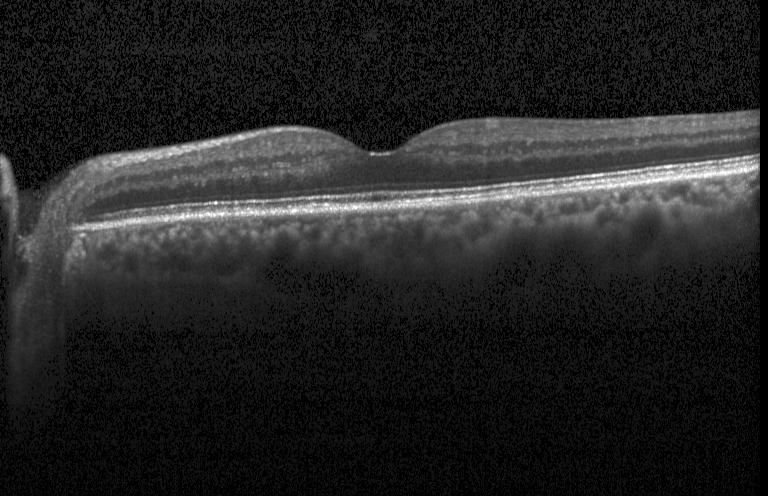 Retinal OCT cross-section
Diagnosis: no evidence of CNV, DME, or drusen.